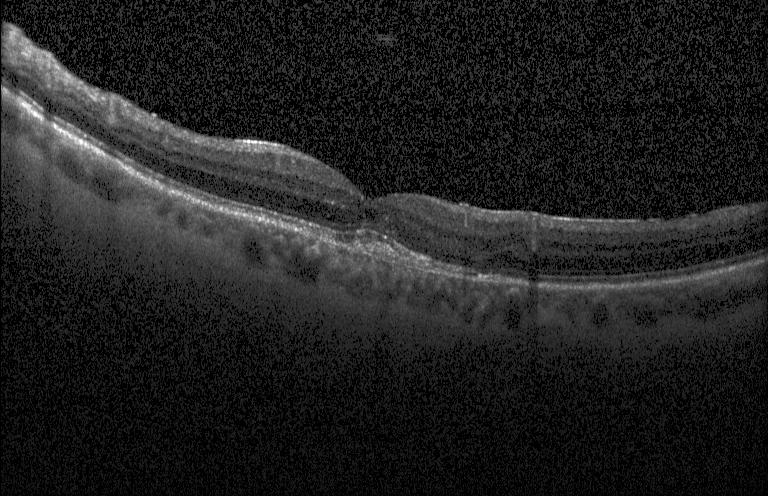

OCT line scan.
Assessment: choroidal neovascularization (CNV).